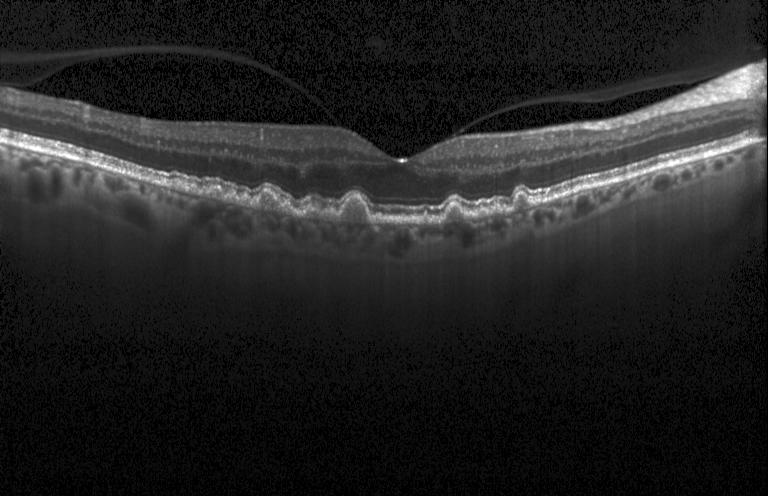
Spectral-domain optical coherence tomography; macular scan; instrument: Heidelberg Spectralis; optical coherence tomography B-scan.
The scan shows drusen.